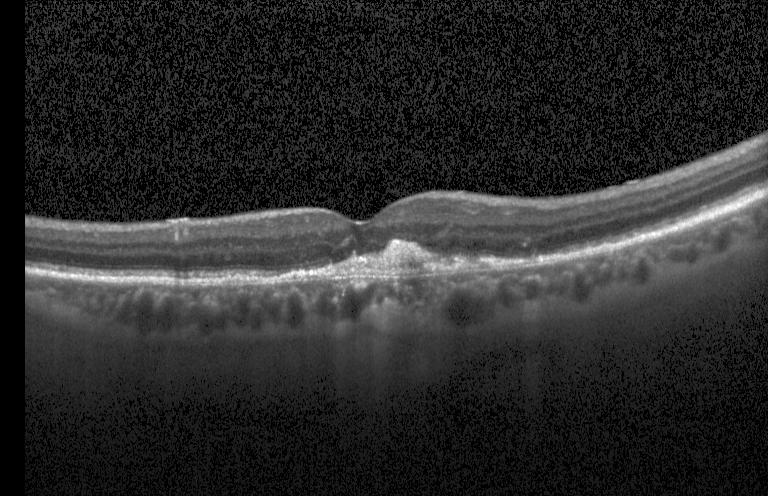

Spectral-domain optical coherence tomography · retinal OCT B-scan.
Assessment: choroidal neovascularization.